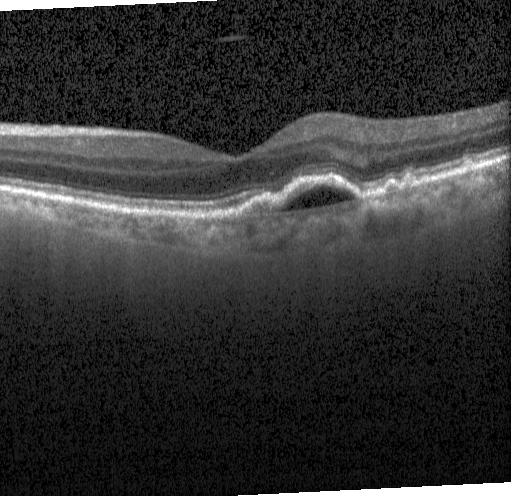
Heidelberg Spectralis OCT system; through the macula; SD-OCT; optical coherence tomography scan. Macular OCT: a choroidal neovascular membrane.